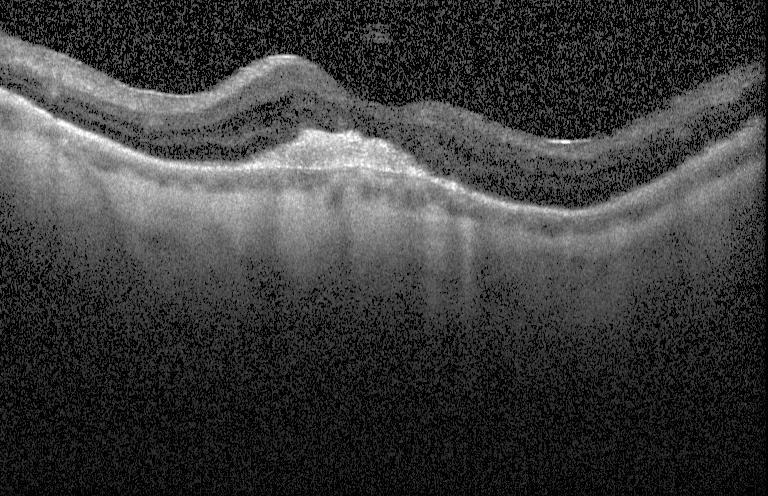 Optical coherence tomography B-scan. Heidelberg Spectralis
Impression: a choroidal neovascular membrane.